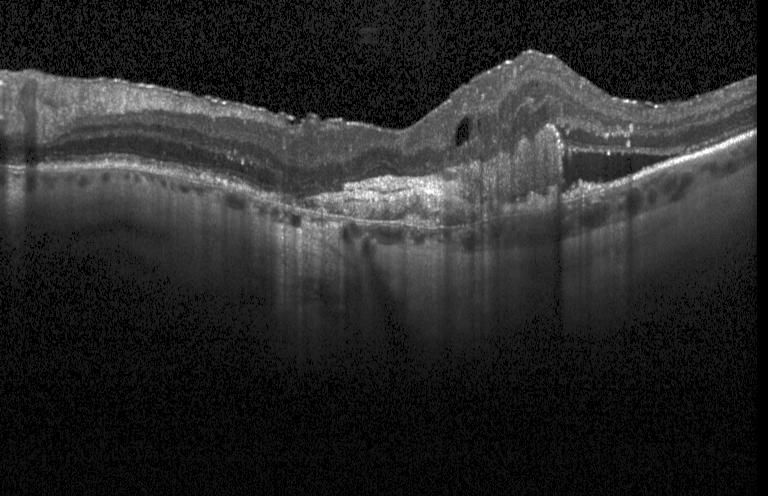

Retinal OCT B-scan; spectral-domain OCT.
Impression: choroidal neovascularization.